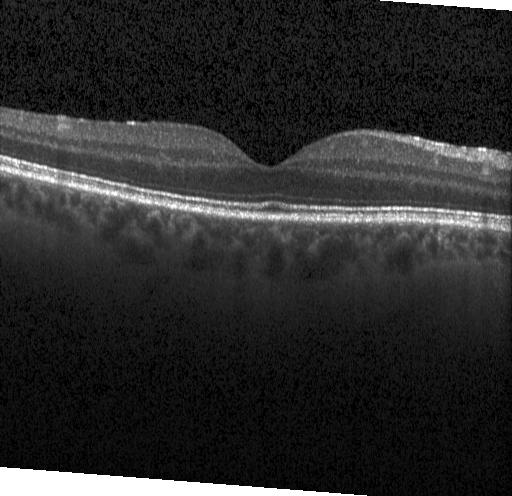 SD-OCT · optical coherence tomography B-scan · Heidelberg Spectralis OCT system · centered on the fovea. Neither choroidal neovascularization, diabetic macular edema, nor drusen.